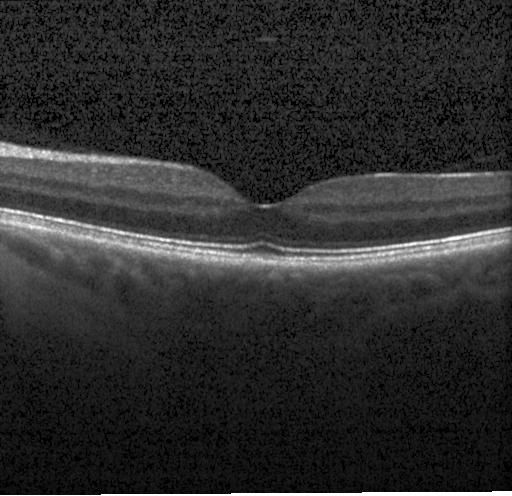
OCT finding: no CNV, no DME, and no drusen.